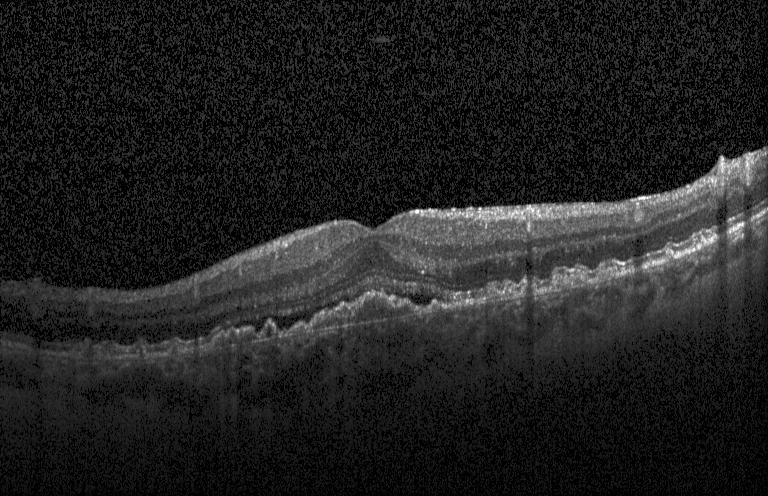
Optical coherence tomography B-scan. Macular scan.
CNV.